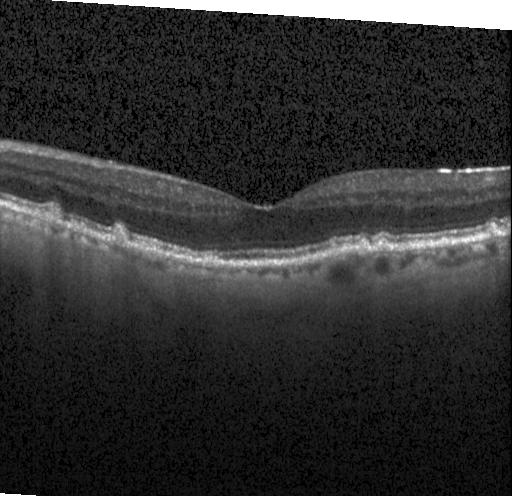

Instrument: Heidelberg Spectralis. SD-OCT. Optical coherence tomography B-scan. Macular scan.
Multiple drusen.